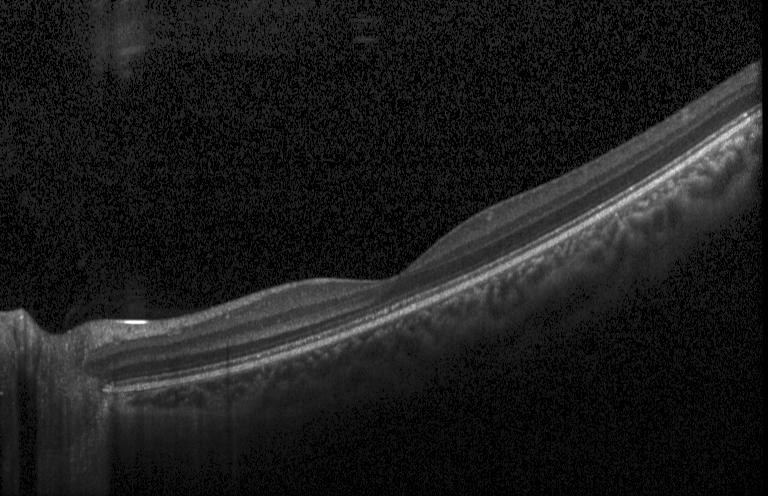
Macular OCT demonstrating no CNV, no DME, and no drusen.